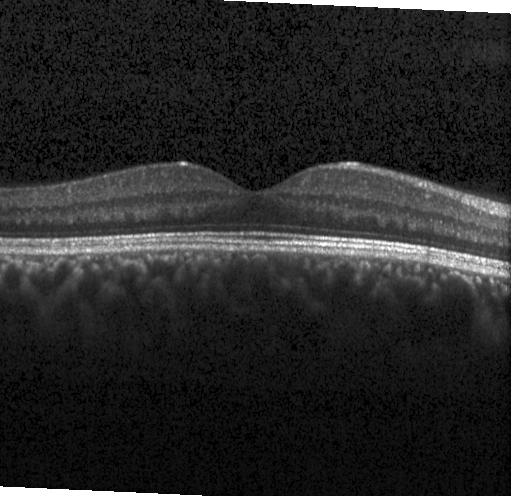

Retinal OCT B-scan.
Diagnosis: no choroidal neovascularization, no diabetic macular edema, and no drusen.